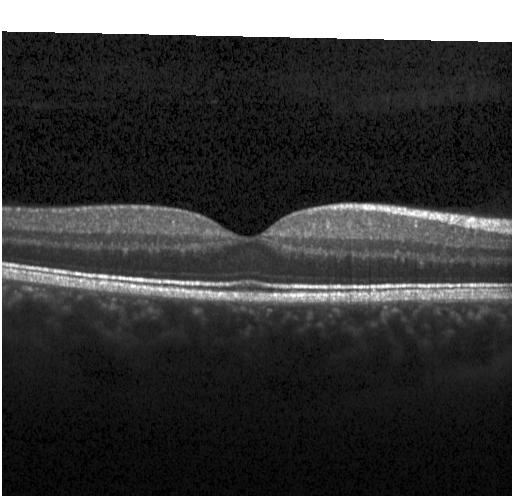 Macular OCT: no choroidal neovascularization, diabetic macular edema, or drusen.